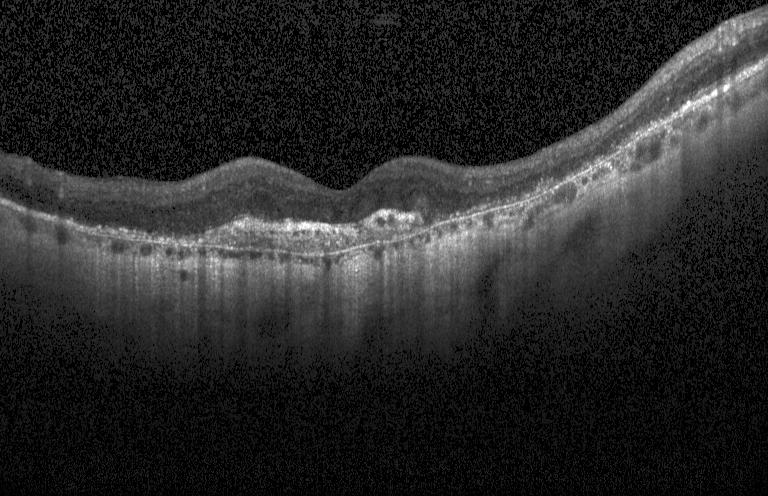

Diagnosis: CNV.